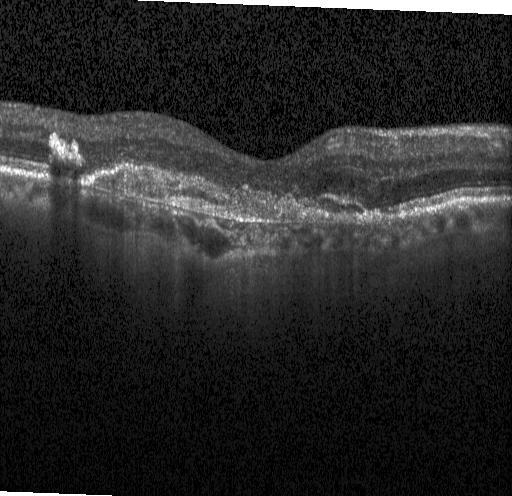
Finding: a choroidal neovascular membrane.